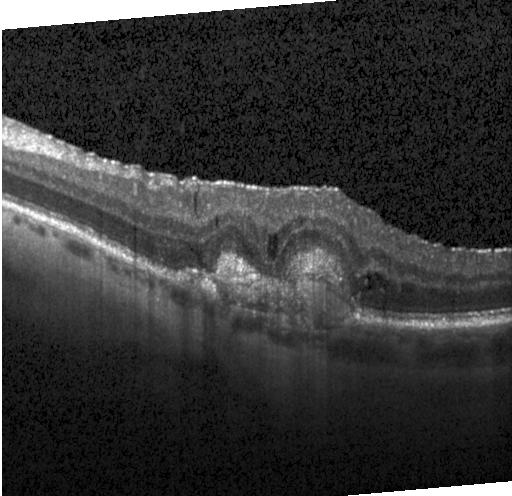
Dx: a choroidal neovascular membrane.